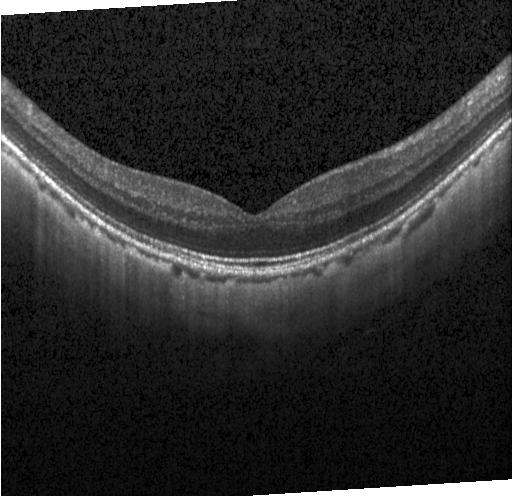
Retinal OCT cross-section · Heidelberg Spectralis · spectral-domain optical coherence tomography · horizontal scan through the fovea
The scan shows no choroidal neovascularization, no diabetic macular edema, and no drusen.